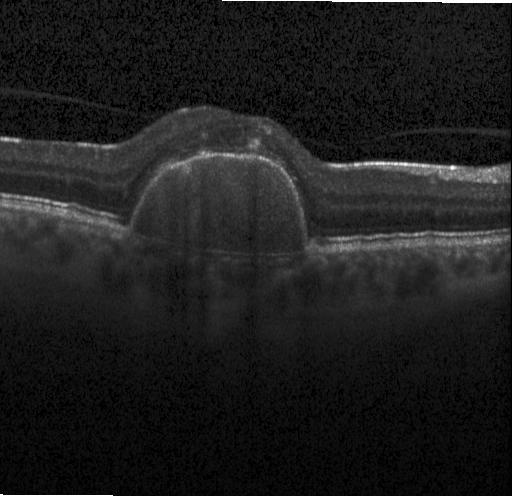

The scan shows a choroidal neovascular membrane.